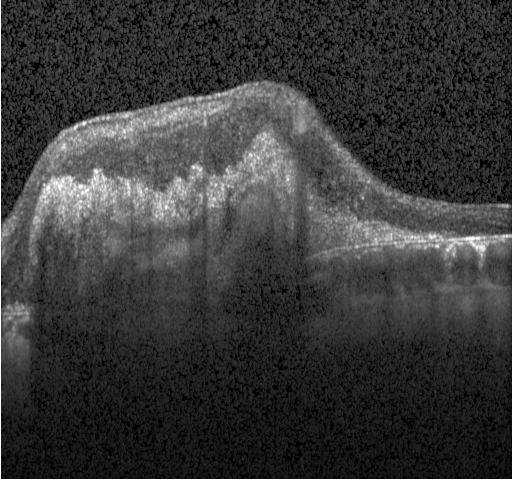

Acquired on a Heidelberg Spectralis, OCT line scan, spectral-domain optical coherence tomography — Diagnosis: CNV.